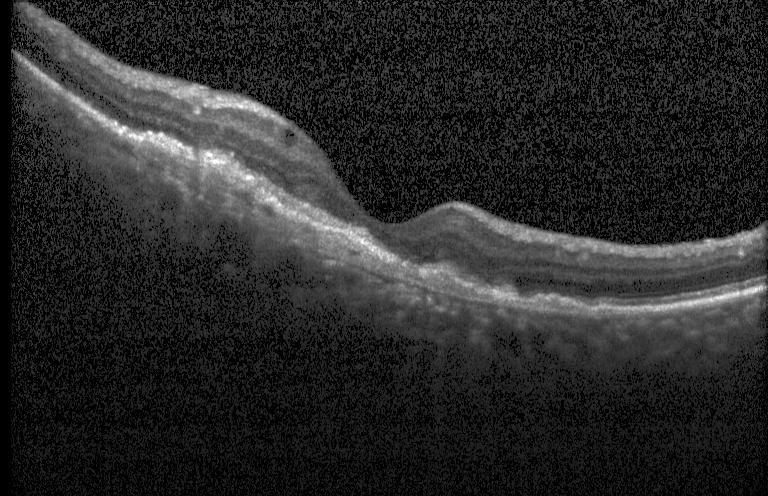
Macular OCT demonstrating choroidal neovascularization.